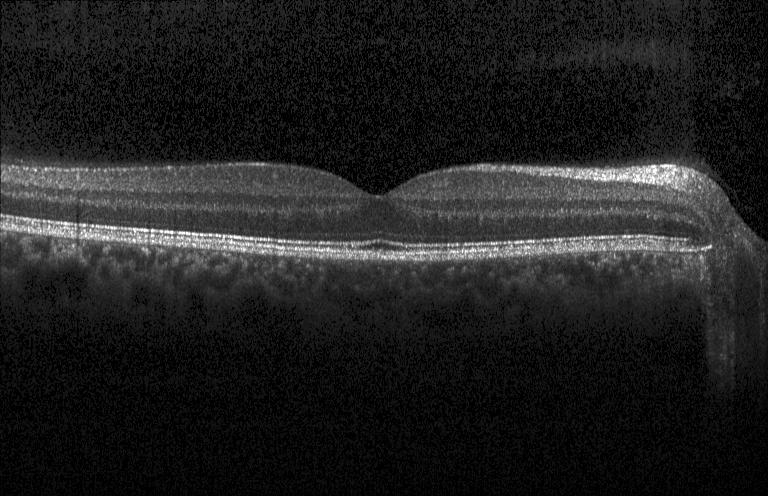

Fovea-centered · instrument: Heidelberg Spectralis · OCT line scan. This B-scan demonstrates no CNV, DME, or drusen.